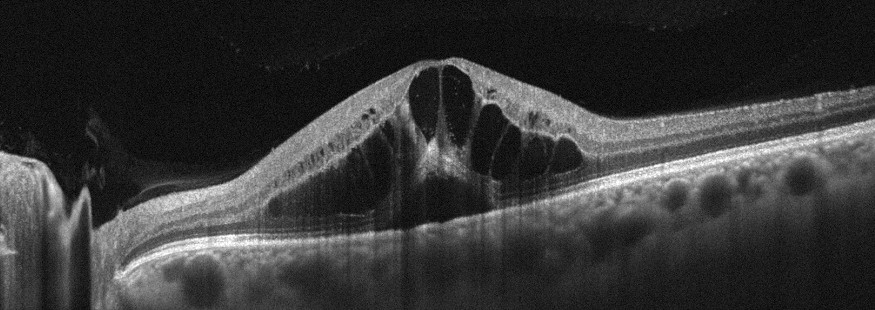

Diagnosis: retinal vein occlusion (RVO).